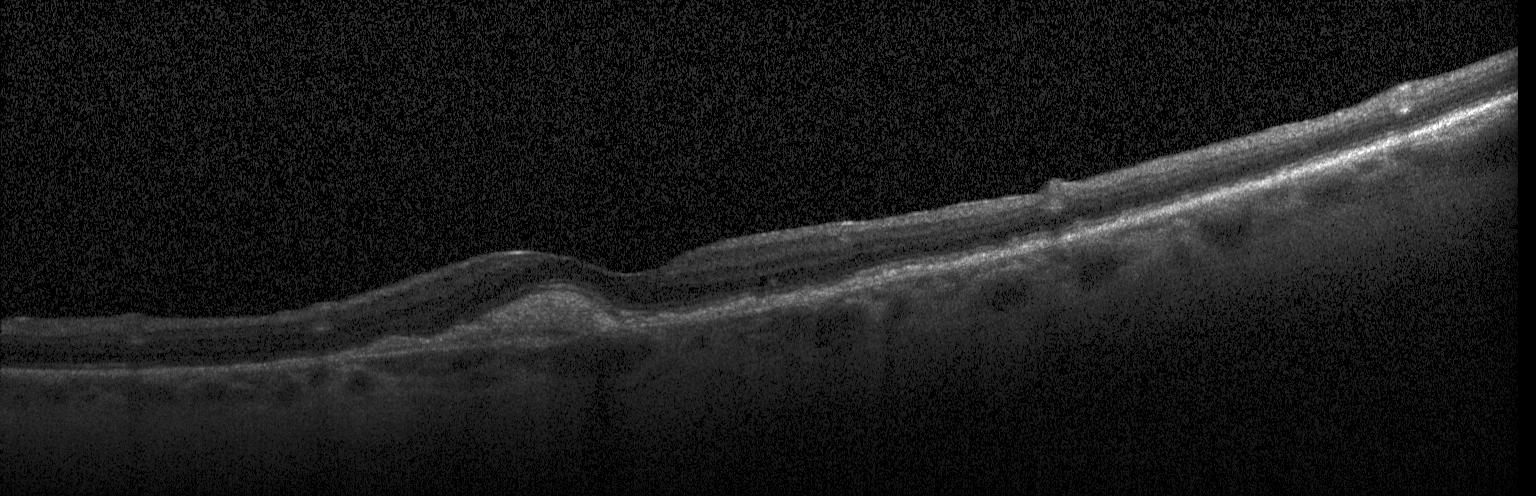
The scan shows choroidal neovascularization (CNV).